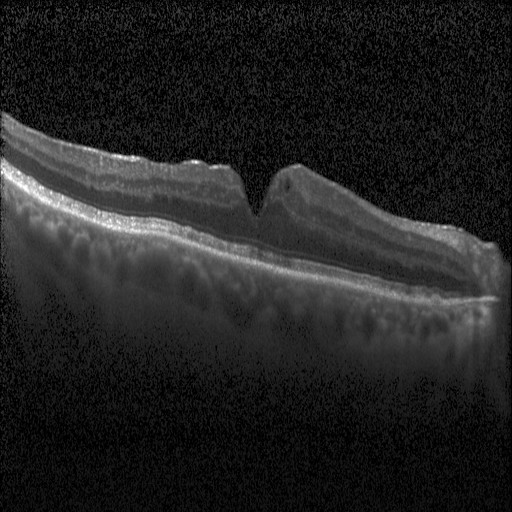

Spectral-domain optical coherence tomography. Optical coherence tomography B-scan. Macular scan. Acquired on a Heidelberg Spectralis
The scan shows diabetic macular edema.